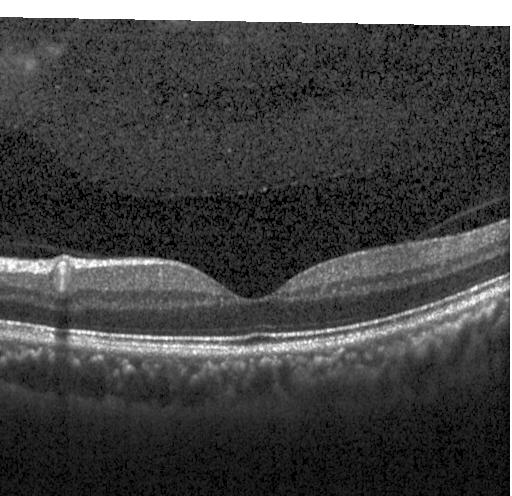

Heidelberg Spectralis OCT system · OCT line scan
Diagnosis: no choroidal neovascularization, no diabetic macular edema, and no drusen.